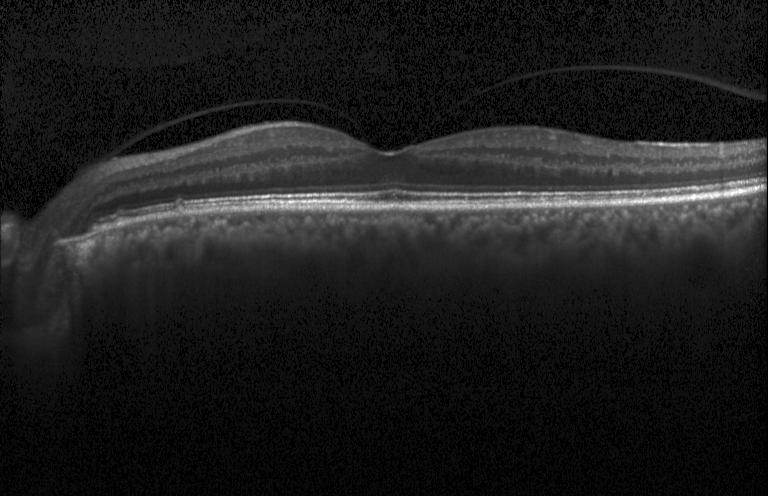 Finding: neither CNV, DME, nor drusen.